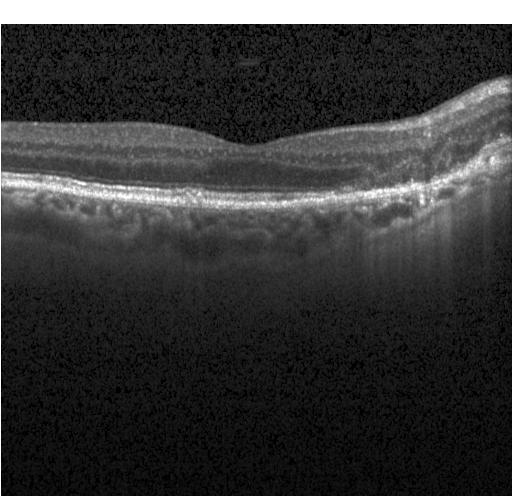

OCT B-scan showing a choroidal neovascular membrane.